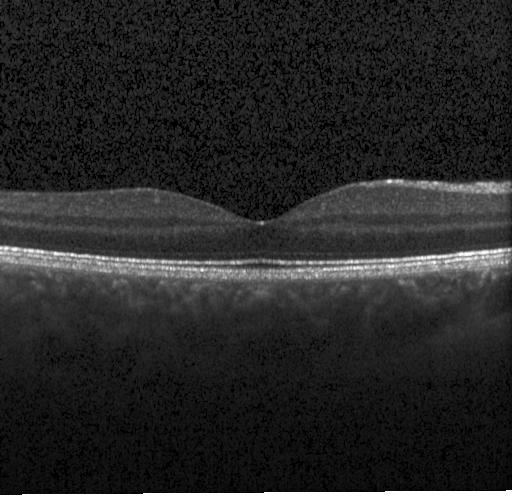
Centered on the fovea · retinal OCT B-scan.
Impression: no evidence of CNV, DME, or drusen.